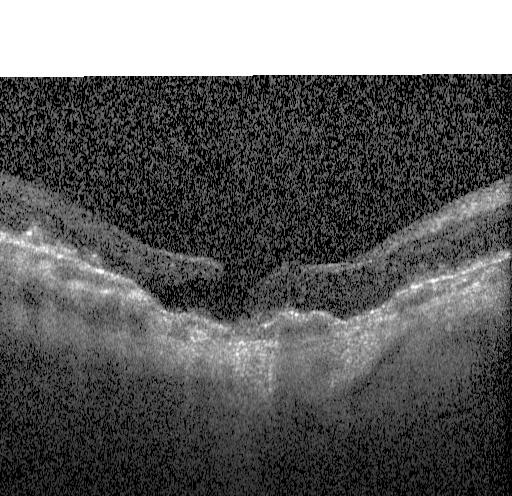

Diagnosis: choroidal neovascularization.